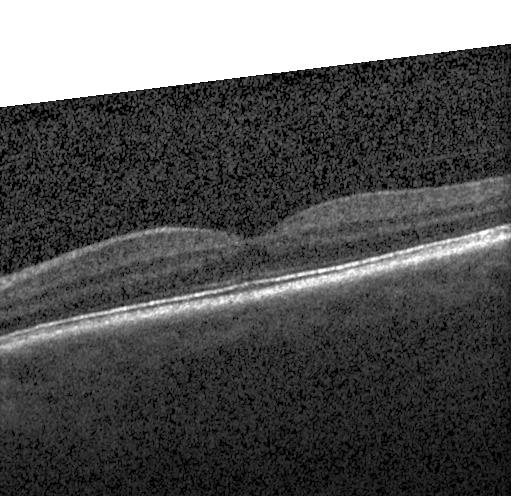 SD-OCT, retinal OCT cross-section, horizontal scan through the fovea
Macular OCT: no choroidal neovascularization, diabetic macular edema, or drusen.